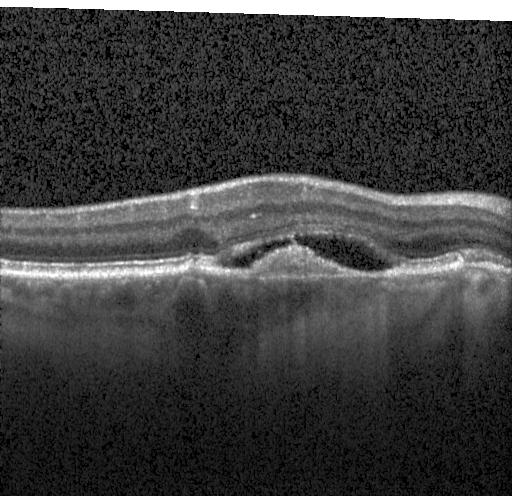

Diagnosis: a choroidal neovascular membrane.